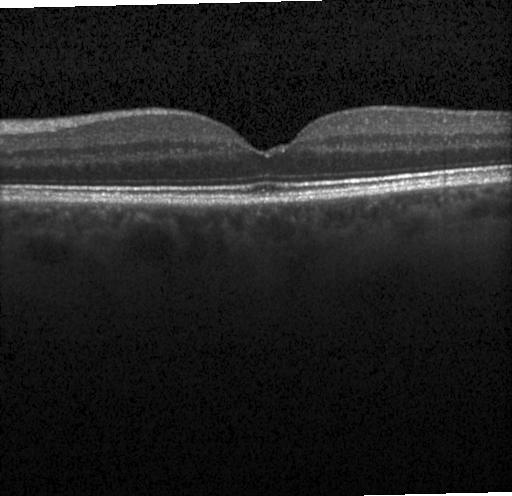 Retinal OCT cross-section showing no choroidal neovascularization, diabetic macular edema, or drusen.